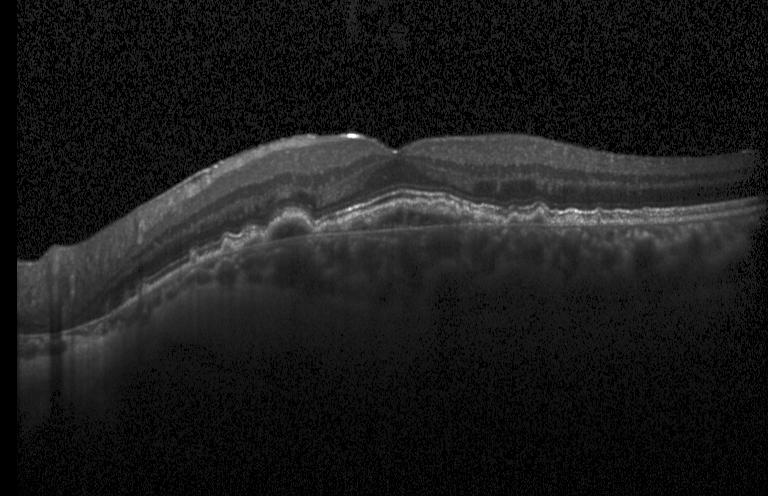
Retinal OCT B-scan — Assessment: choroidal neovascularization.